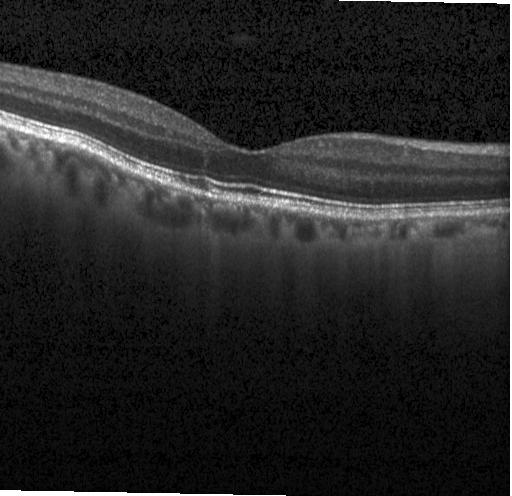

Instrument: Heidelberg Spectralis; OCT B-scan; centered on the fovea — No choroidal neovascularization, no diabetic macular edema, and no drusen.